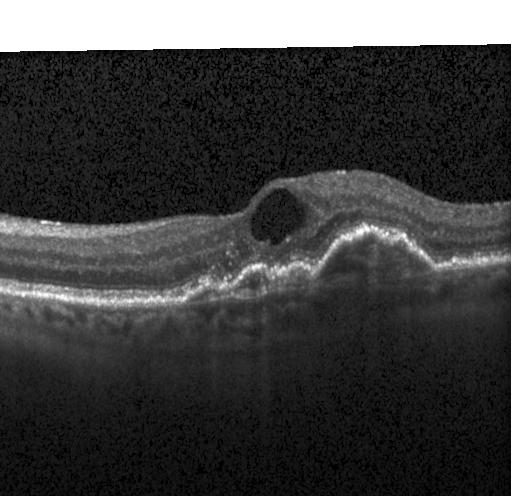 Instrument: Heidelberg Spectralis · macular scan · spectral-domain OCT · optical coherence tomography scan. Impression: a choroidal neovascular membrane.